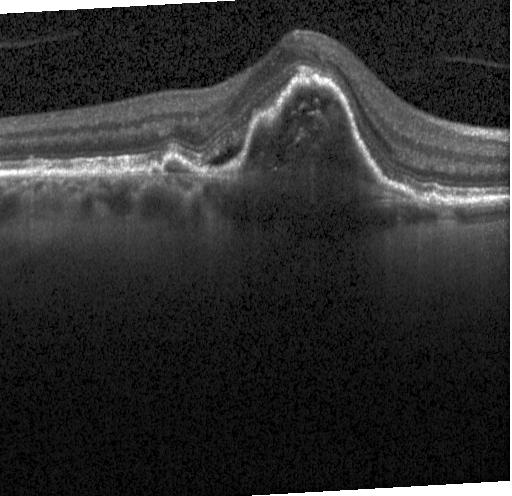 OCT B-scan showing a choroidal neovascular membrane.